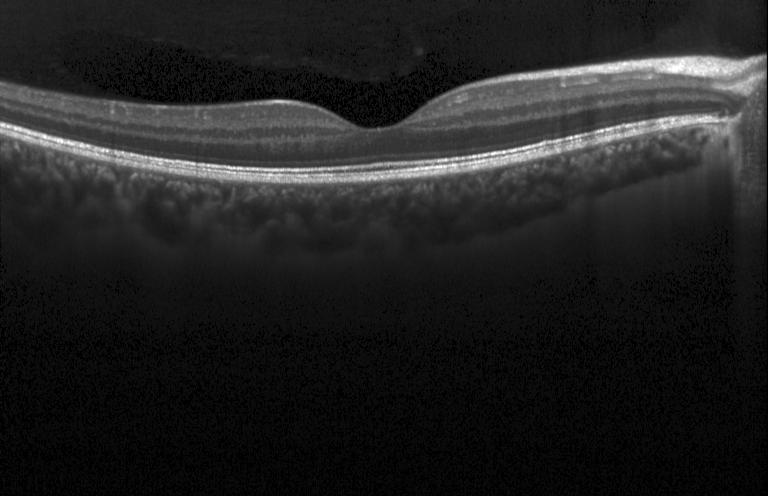 Heidelberg Spectralis OCT system · spectral-domain OCT · optical coherence tomography scan
Finding: neither choroidal neovascularization, diabetic macular edema, nor drusen.